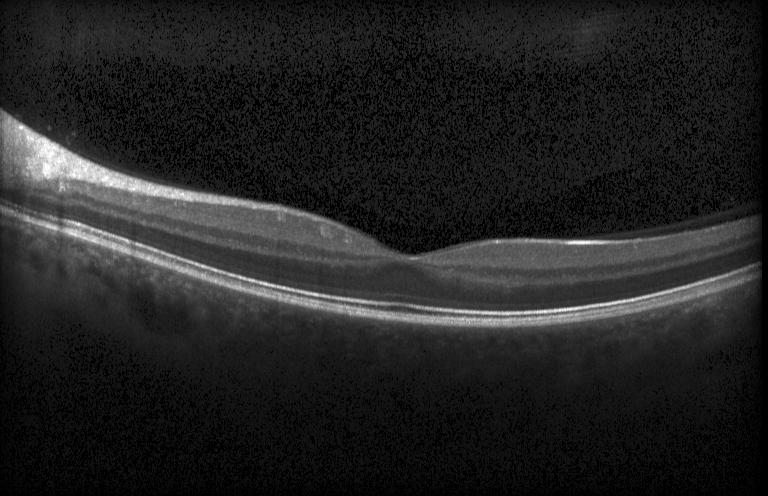
Spectral-domain optical coherence tomography. Retinal OCT B-scan. Diagnosis: no choroidal neovascularization, diabetic macular edema, or drusen.